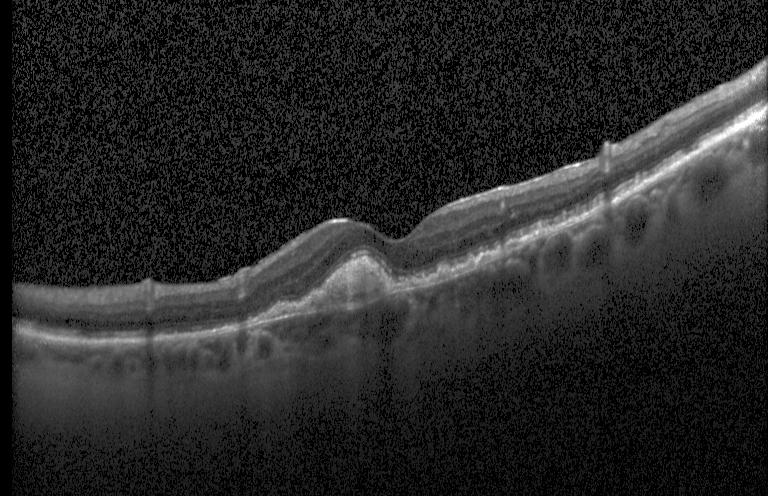

OCT finding: a choroidal neovascular membrane.